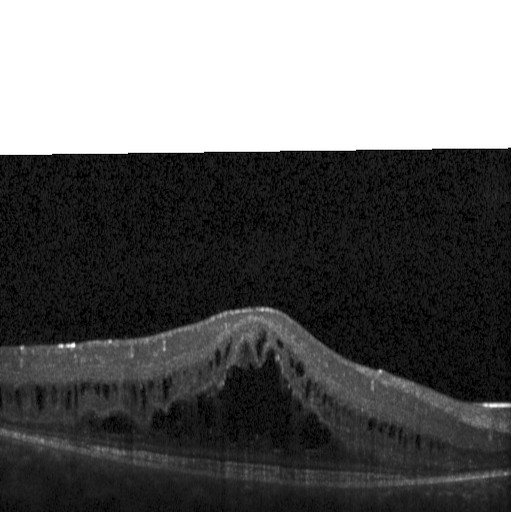 OCT finding: DME.